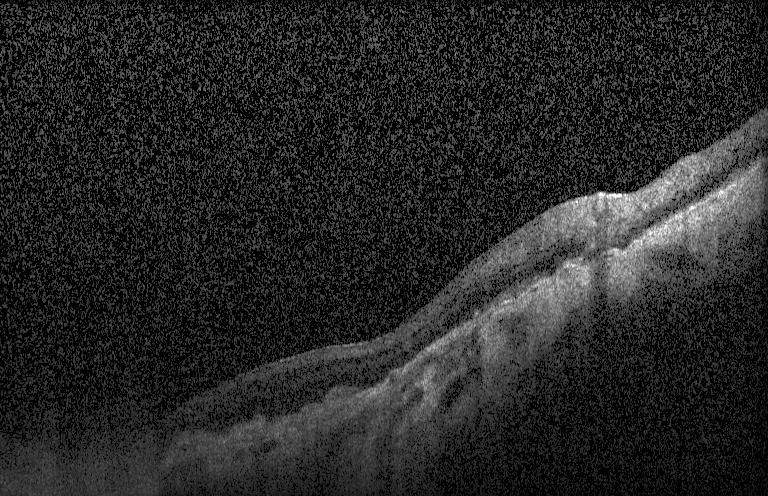
Optical coherence tomography scan; spectral-domain optical coherence tomography; fovea-centered
Assessment: CNV.